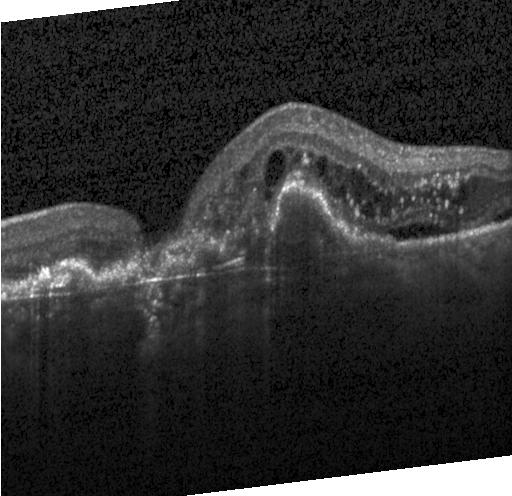 Macular OCT: a choroidal neovascular membrane.